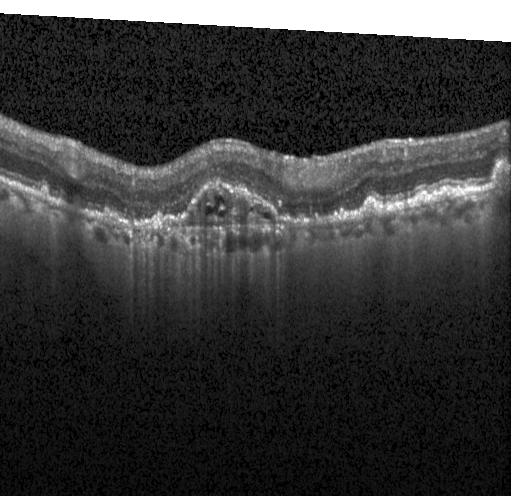

Spectral-domain optical coherence tomography; optical coherence tomography B-scan. Dx: a choroidal neovascular membrane.